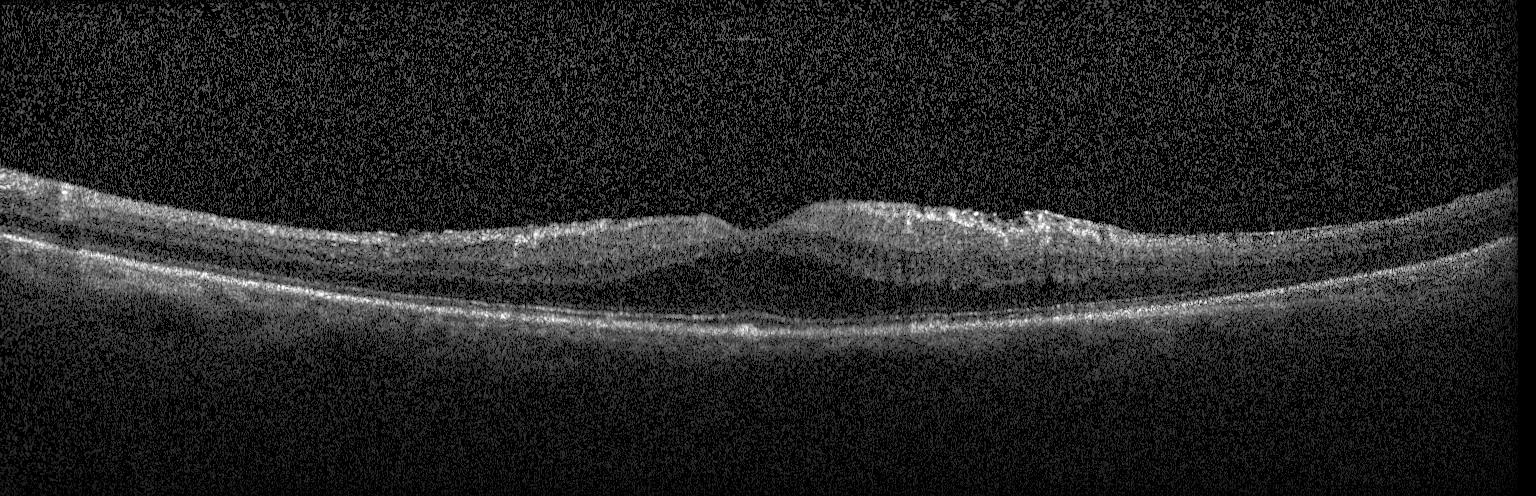 Impression: diabetic macular edema.